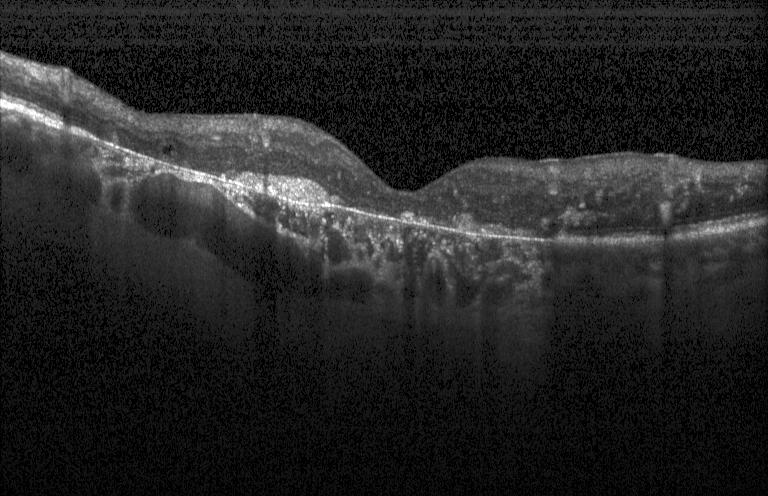
OCT B-scan.
Diagnosis: CNV.